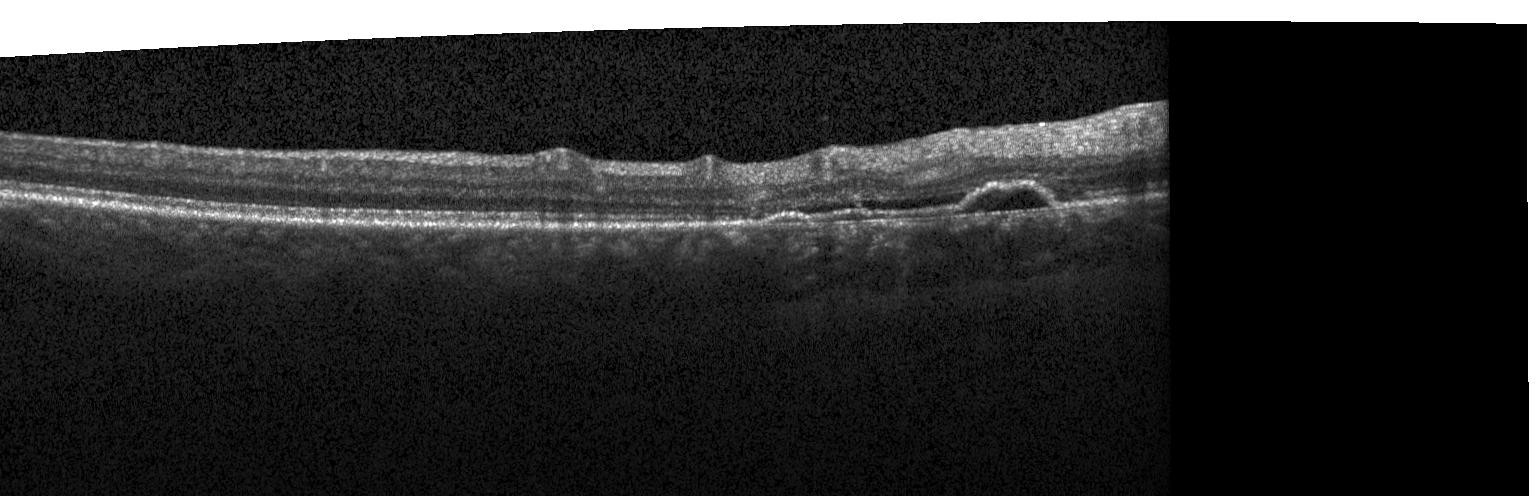

Heidelberg Spectralis OCT system · optical coherence tomography B-scan
OCT finding: CNV.